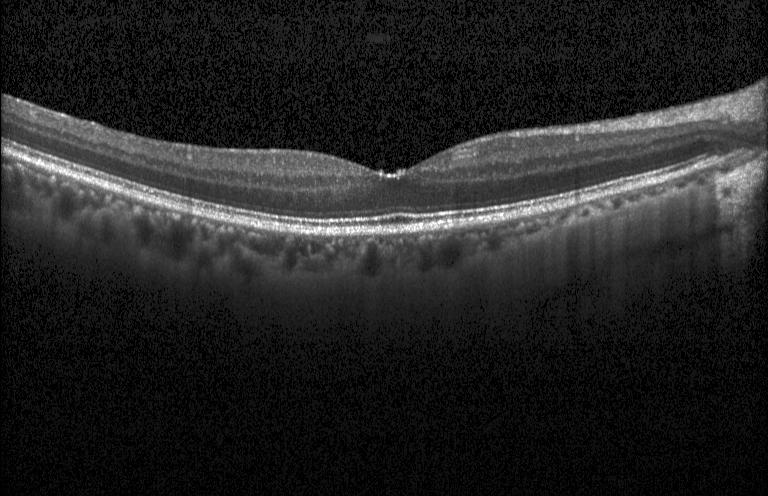 OCT finding: no choroidal neovascularization, diabetic macular edema, or drusen.